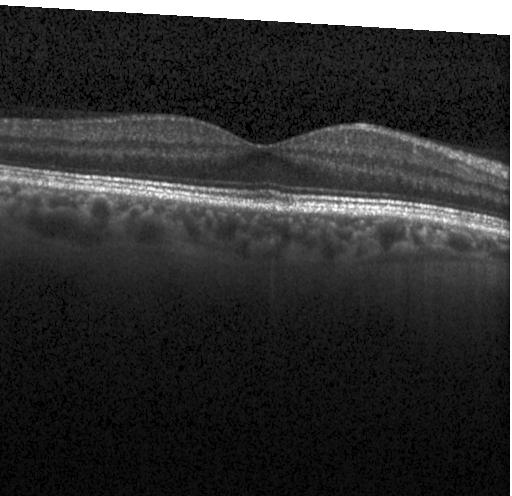
Dx: no evidence of CNV, DME, or drusen.